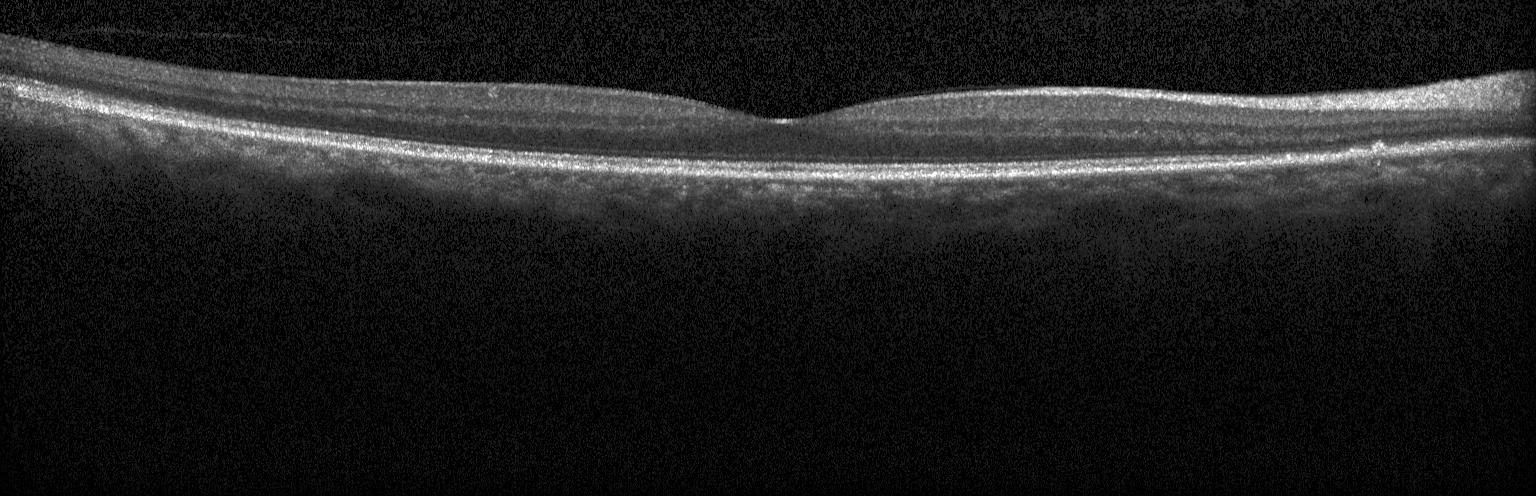

Heidelberg Spectralis OCT system · optical coherence tomography B-scan. Assessment: no evidence of choroidal neovascularization, diabetic macular edema, or drusen.